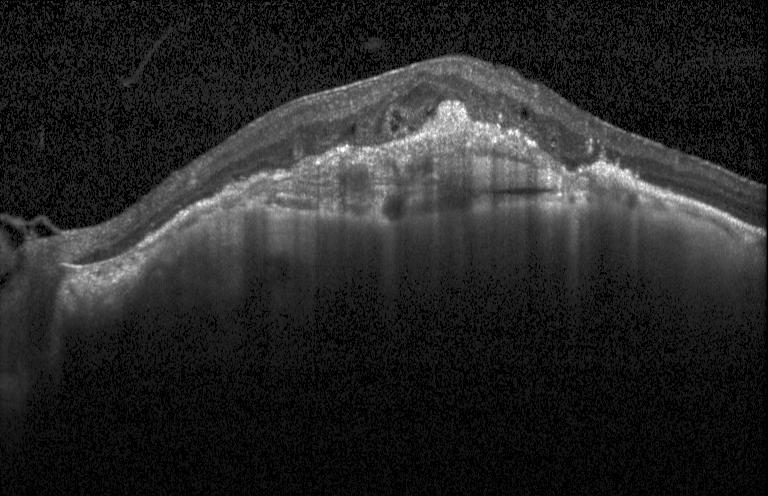

Optical coherence tomography scan.
Macular OCT: choroidal neovascularization.